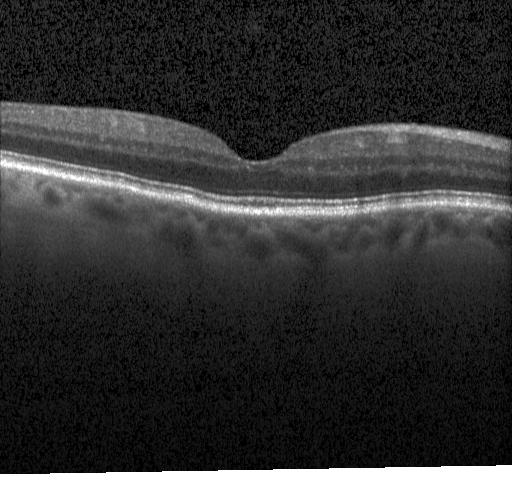 Spectral-domain OCT B-scan: no CNV, DME, or drusen.